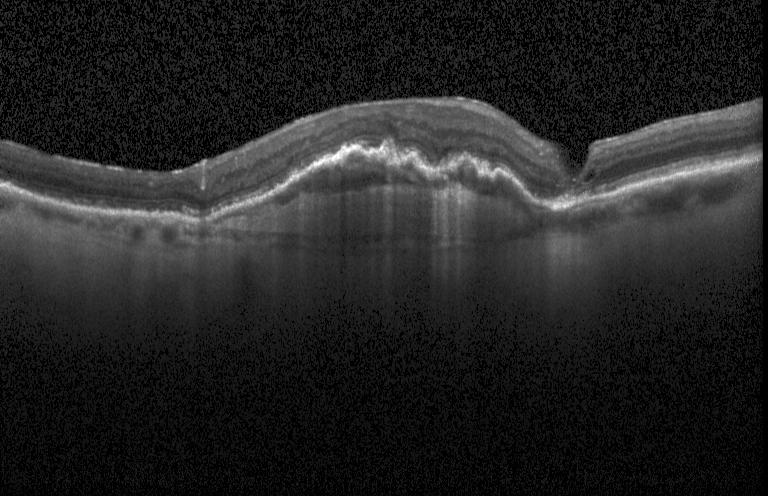
Macular scan · Heidelberg Spectralis OCT system · optical coherence tomography scan. Impression: CNV.